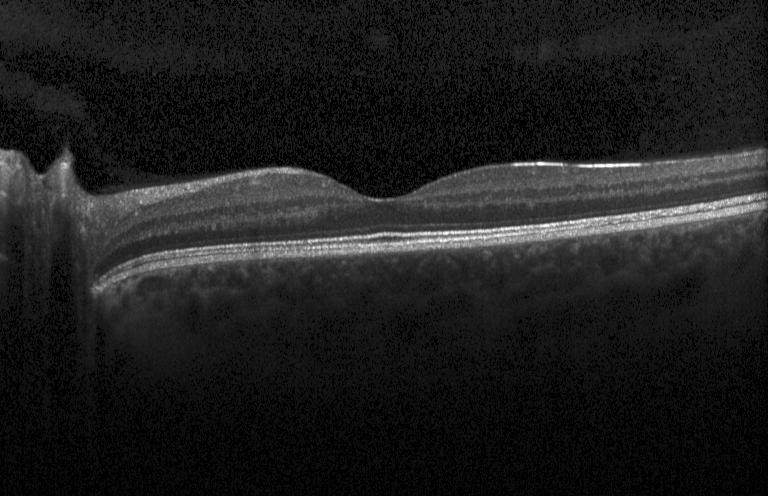
OCT finding: no CNV, no DME, and no drusen.